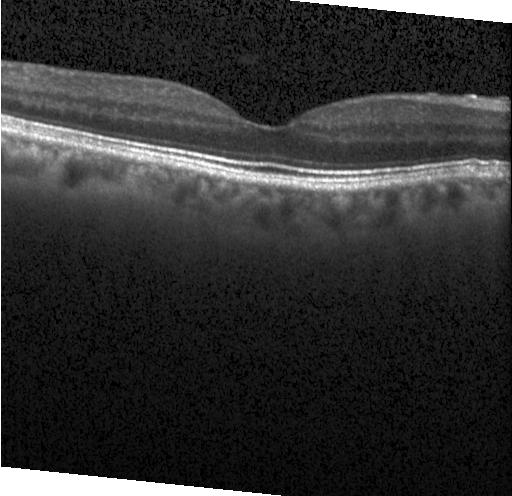
Heidelberg Spectralis OCT system; horizontal scan through the fovea; spectral-domain optical coherence tomography; retinal OCT B-scan
Finding: neither CNV, DME, nor drusen.